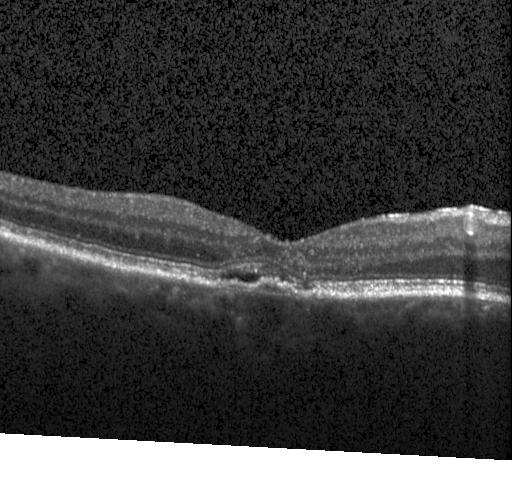 OCT B-scan — Finding: a choroidal neovascular membrane.